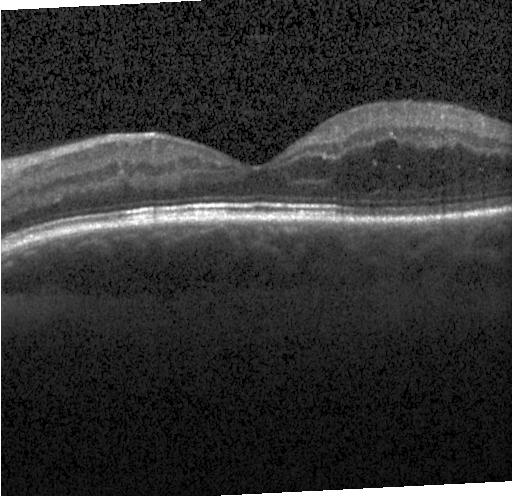 Dx: DME.